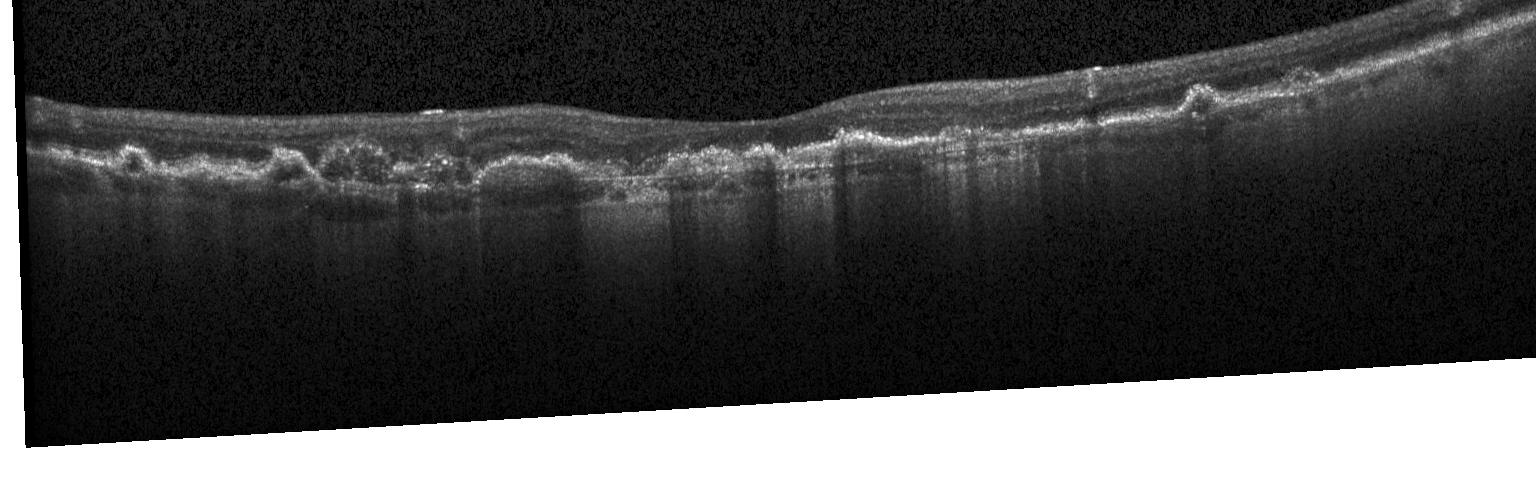
Optical coherence tomography scan — Impression: a choroidal neovascular membrane.